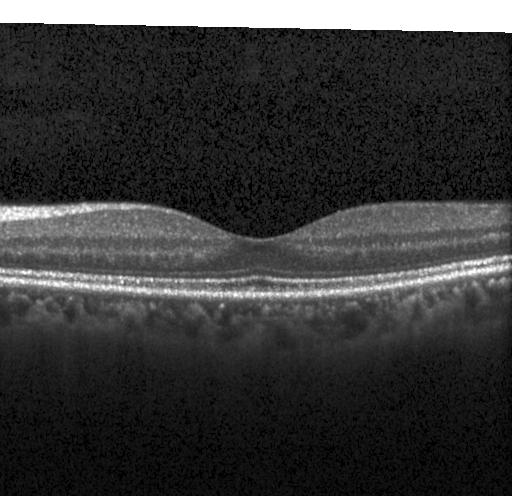

Retinal OCT B-scan, spectral-domain optical coherence tomography. Dx: neither CNV, DME, nor drusen.